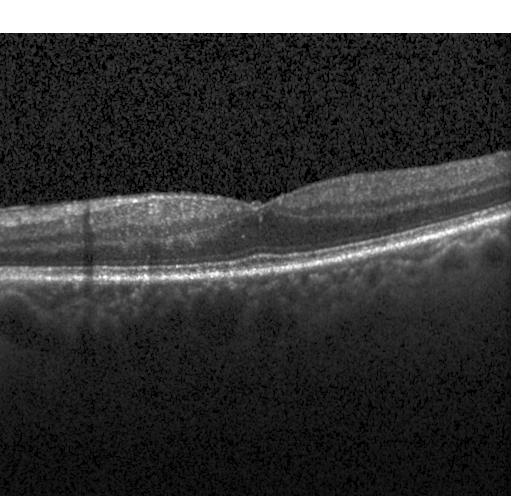

Retinal OCT B-scan. Macular OCT: no choroidal neovascularization, diabetic macular edema, or drusen.